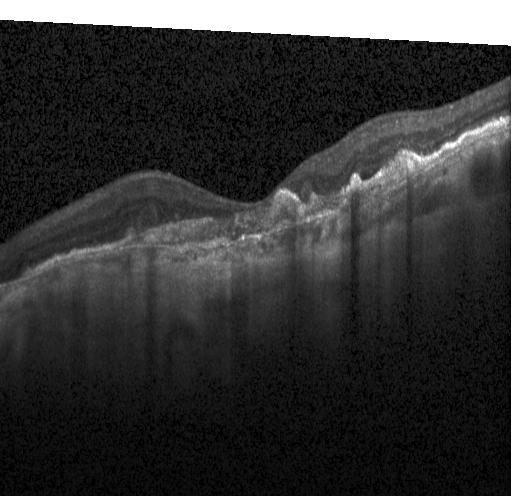 Dx: choroidal neovascularization.